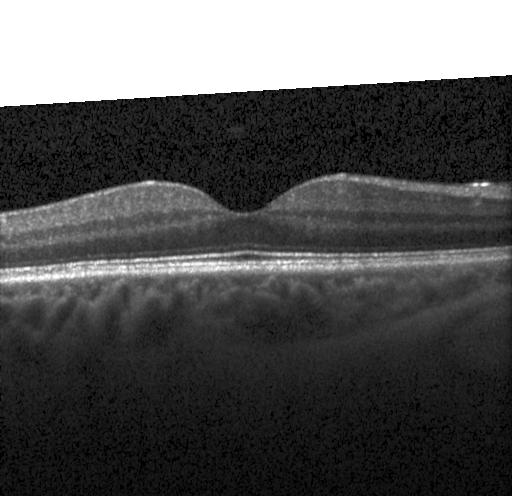 Centered on the fovea · spectral-domain optical coherence tomography · instrument: Heidelberg Spectralis · OCT line scan — The scan shows neither choroidal neovascularization, diabetic macular edema, nor drusen.